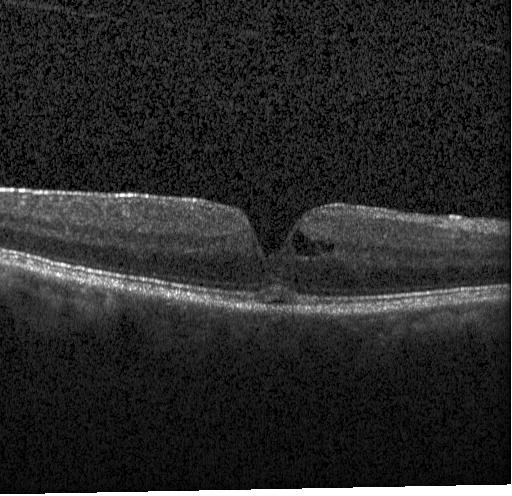
Finding: diabetic macular edema.